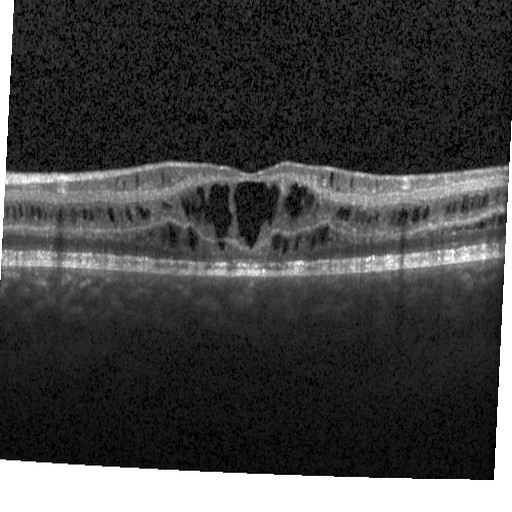
Macular scan · retinal OCT cross-section.
DME.